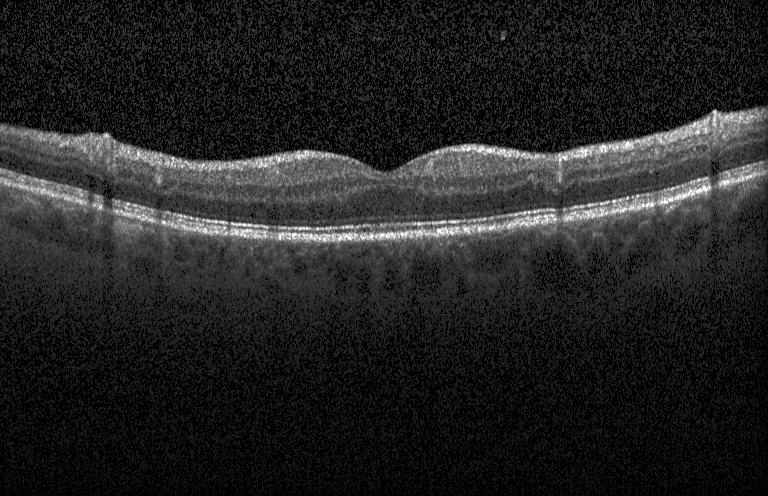 Impression: no choroidal neovascularization, no diabetic macular edema, and no drusen.